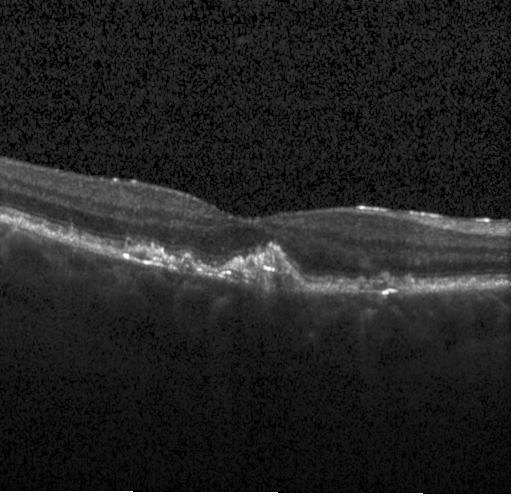
Retinal OCT cross-section.
The scan shows choroidal neovascularization (CNV).